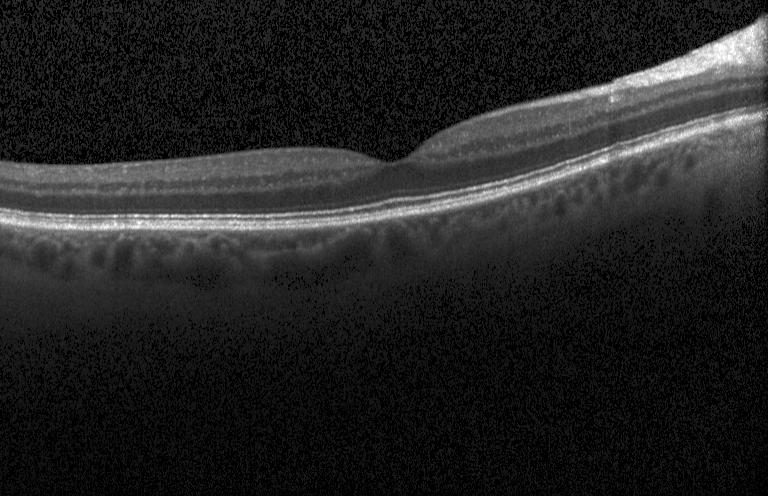
Retinal OCT cross-section showing no choroidal neovascularization, no diabetic macular edema, and no drusen.